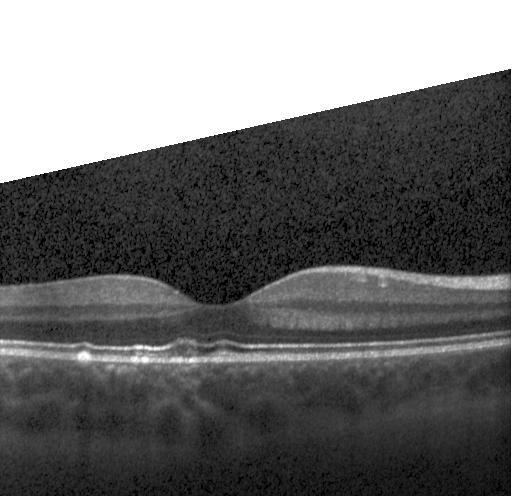
Heidelberg Spectralis, spectral-domain optical coherence tomography, optical coherence tomography B-scan, fovea-centered.
Finding: sub-RPE drusenoid deposits.